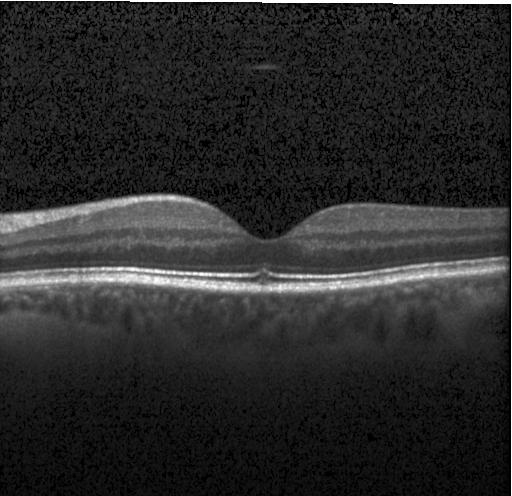

SD-OCT · optical coherence tomography scan. Finding: neither choroidal neovascularization, diabetic macular edema, nor drusen.